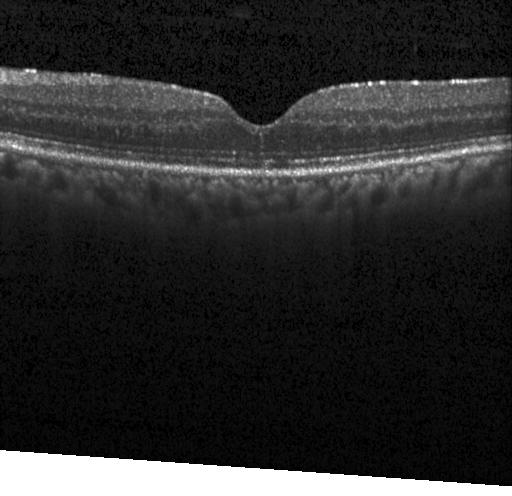
OCT line scan · spectral-domain optical coherence tomography
This B-scan demonstrates no choroidal neovascularization, no diabetic macular edema, and no drusen.